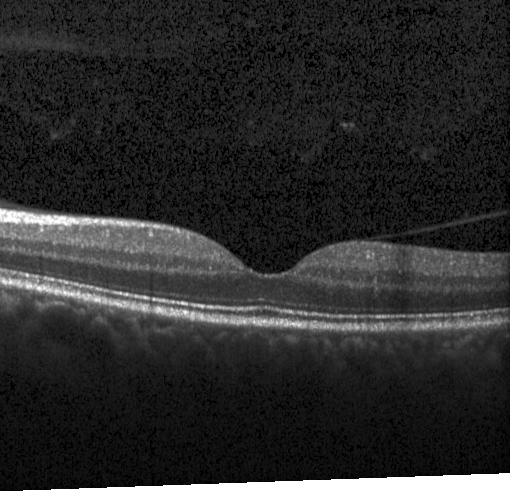

Macular OCT demonstrating no choroidal neovascularization, diabetic macular edema, or drusen.